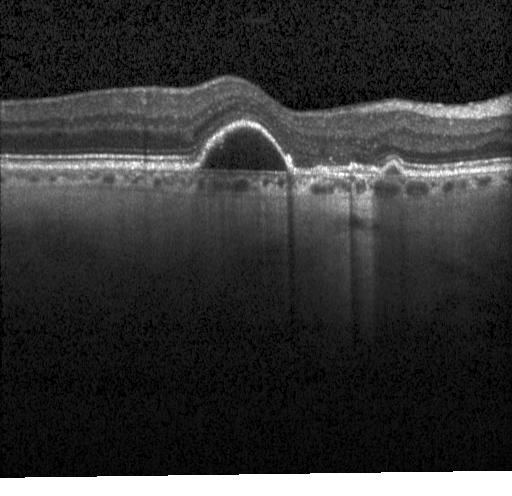 OCT scan showing choroidal neovascularization (CNV).